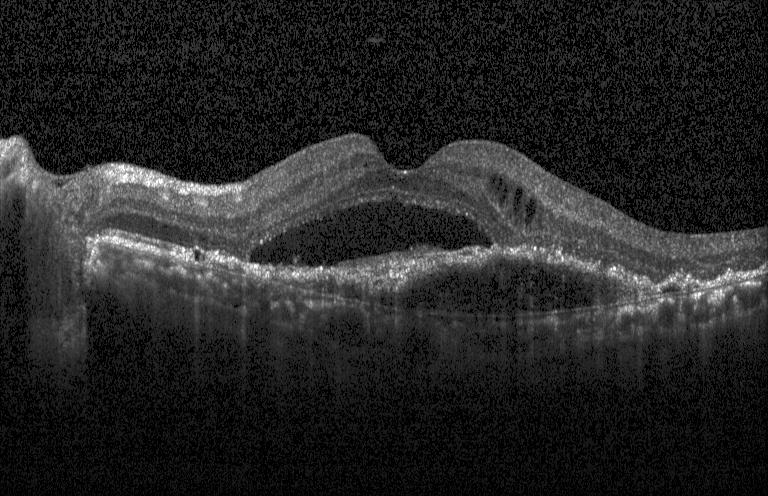 Retinal OCT cross-section · centered on the fovea · instrument: Heidelberg Spectralis — Diagnosis: CNV.